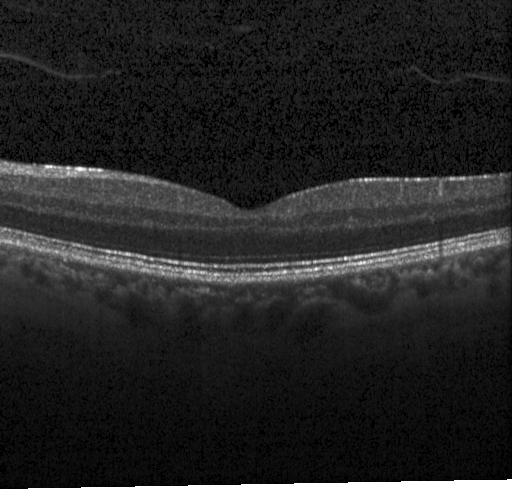
The scan shows no CNV, DME, or drusen.